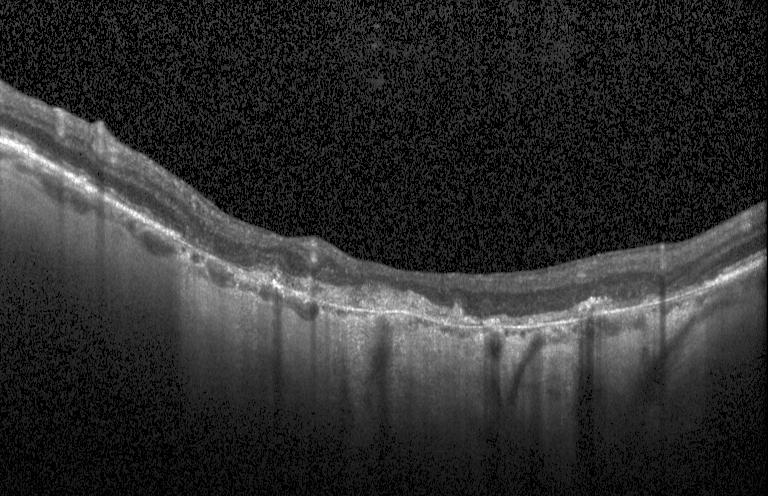

Finding: a choroidal neovascular membrane.